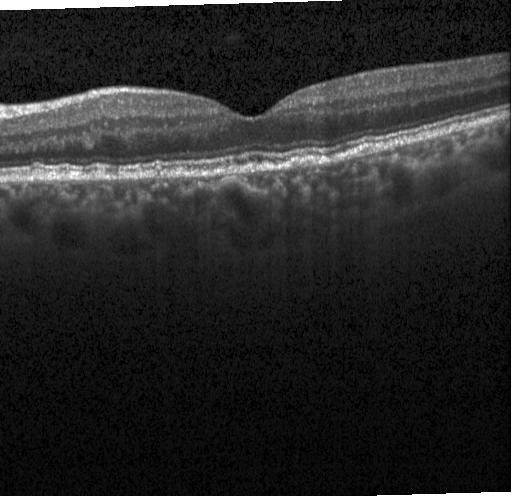

Horizontal scan through the fovea, OCT line scan. Assessment: sub-RPE drusenoid deposits.